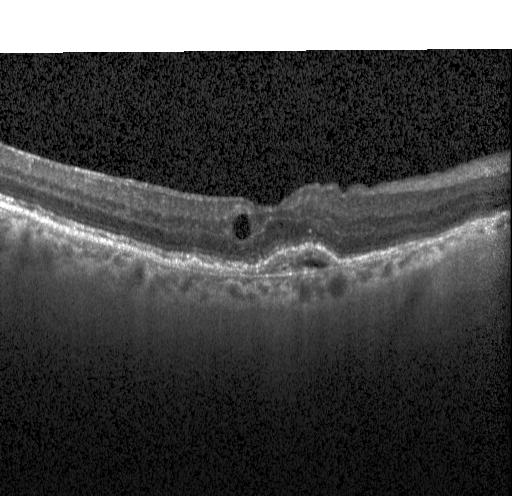

Through the macula, spectral-domain OCT, optical coherence tomography scan — Dx: CNV.